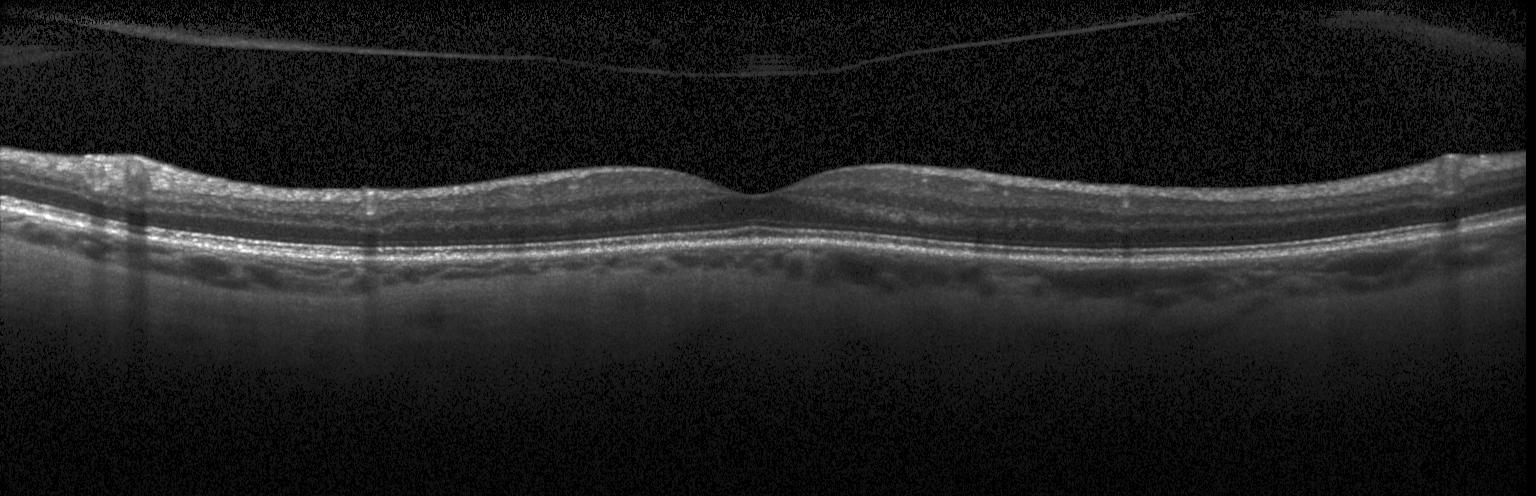 OCT B-scan · SD-OCT · horizontal scan through the fovea · Heidelberg Spectralis OCT system
OCT finding: no choroidal neovascularization, no diabetic macular edema, and no drusen.